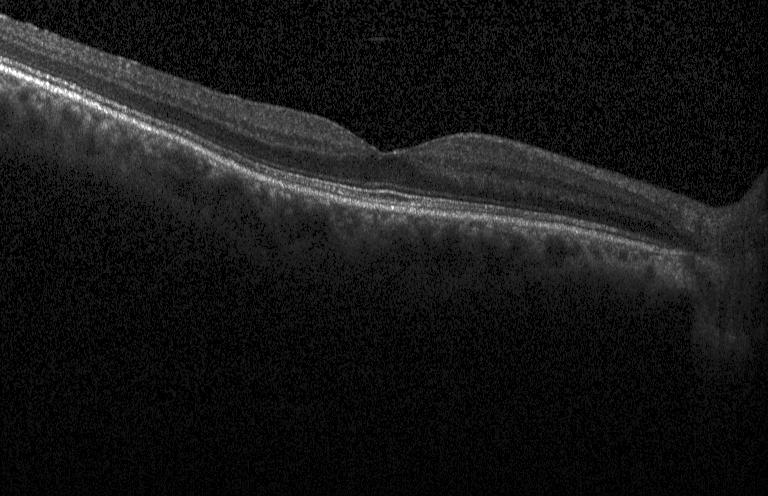
Optical coherence tomography B-scan. Finding: neither choroidal neovascularization, diabetic macular edema, nor drusen.